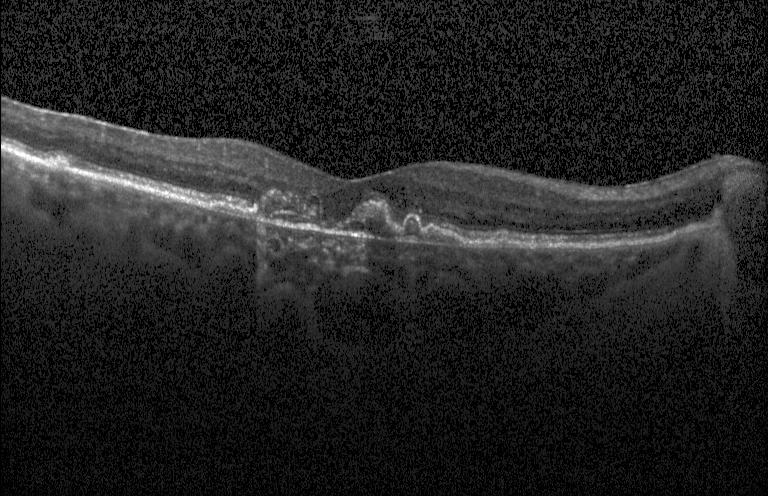

OCT B-scan · Heidelberg Spectralis · through the macula · spectral-domain OCT. Impression: CNV.